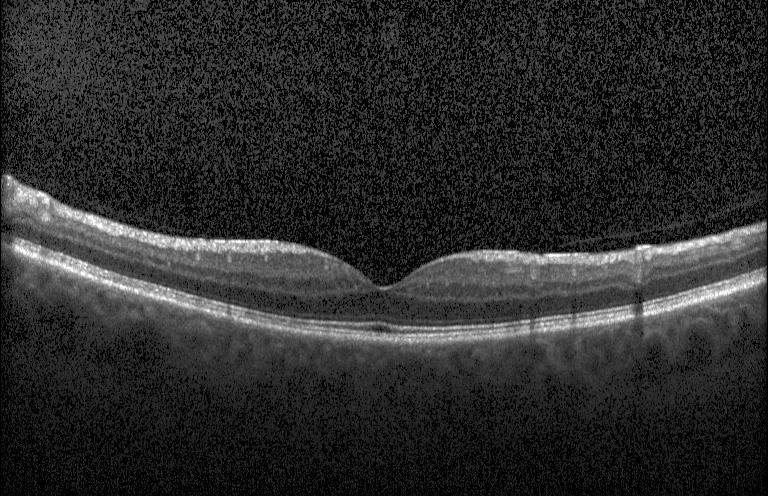
Optical coherence tomography scan. Spectral-domain OCT. This B-scan demonstrates no evidence of CNV, DME, or drusen.